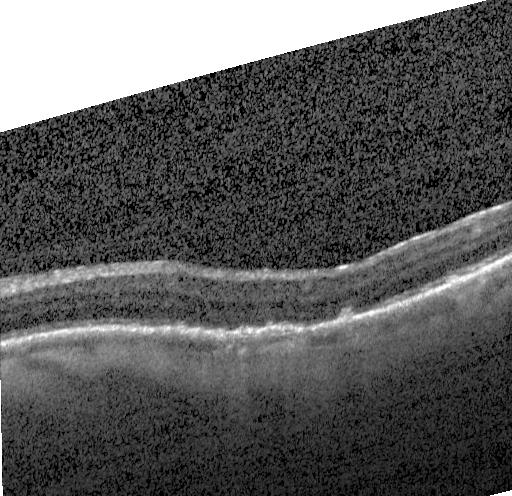
Macular scan, retinal OCT B-scan, instrument: Heidelberg Spectralis
Finding: sub-RPE drusenoid deposits.